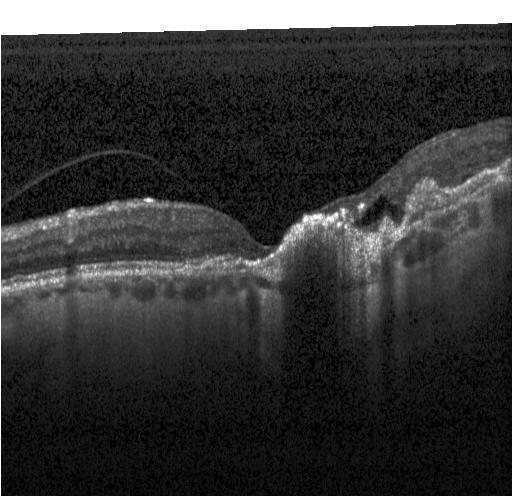 Optical coherence tomography B-scan; spectral-domain optical coherence tomography; centered on the fovea; instrument: Heidelberg Spectralis. Finding: a choroidal neovascular membrane.